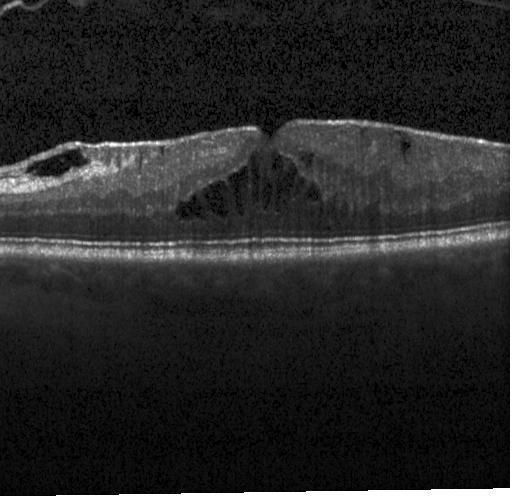
Optical coherence tomography B-scan.
Macular OCT: diabetic macular edema (DME).